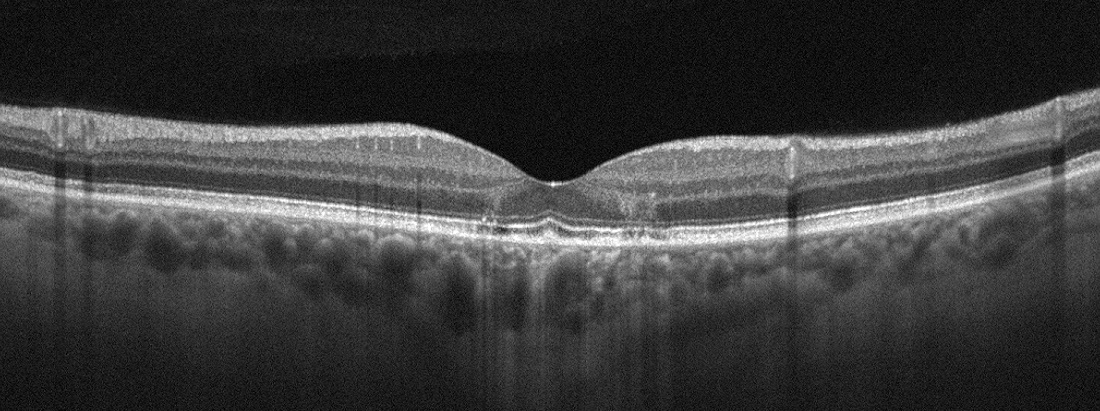
The scan shows age-related macular degeneration (AMD).